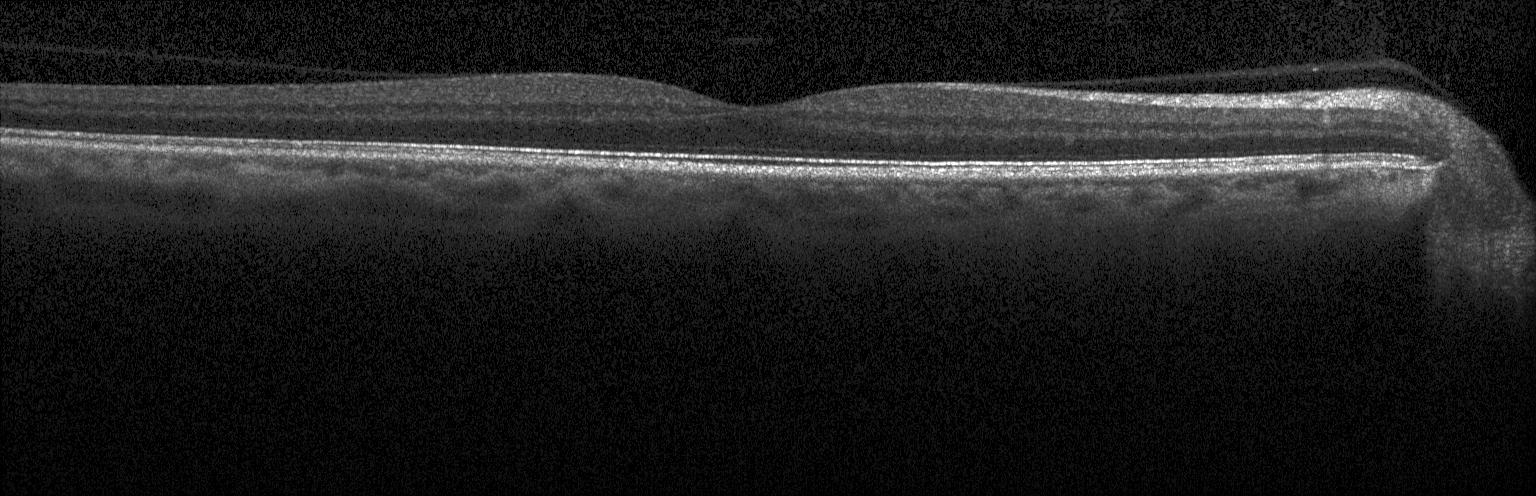
OCT line scan; Heidelberg Spectralis OCT system; horizontal scan through the fovea; spectral-domain optical coherence tomography.
Macular OCT: no choroidal neovascularization, diabetic macular edema, or drusen.